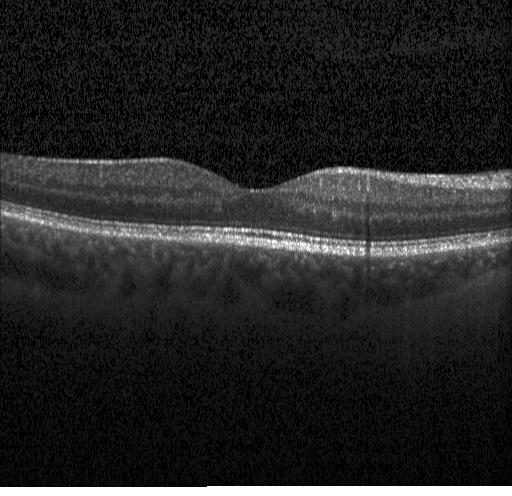 Optical coherence tomography scan. Through the macula. Instrument: Heidelberg Spectralis — Neither CNV, DME, nor drusen.